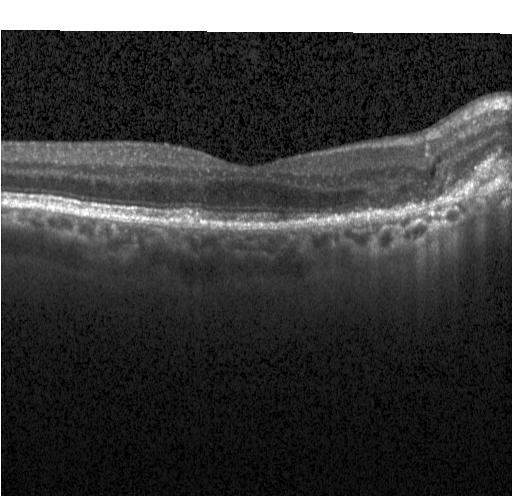
Macular OCT: a choroidal neovascular membrane.